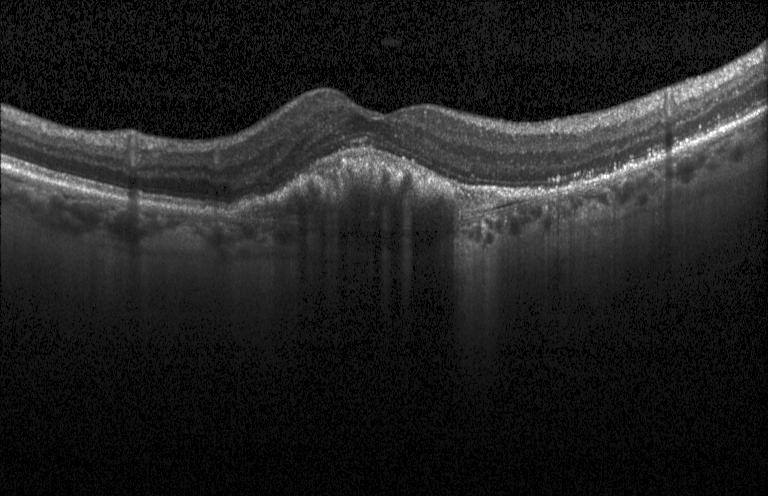 Finding: a choroidal neovascular membrane.